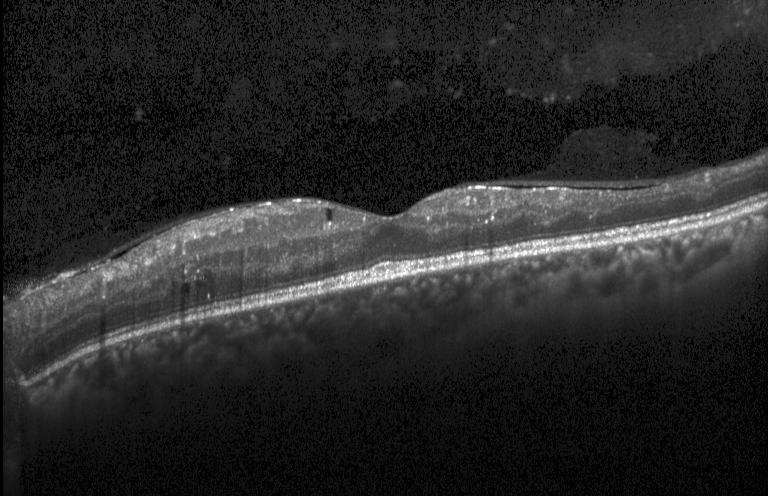
Retinal OCT B-scan, centered on the fovea — Diagnosis: diabetic macular edema.